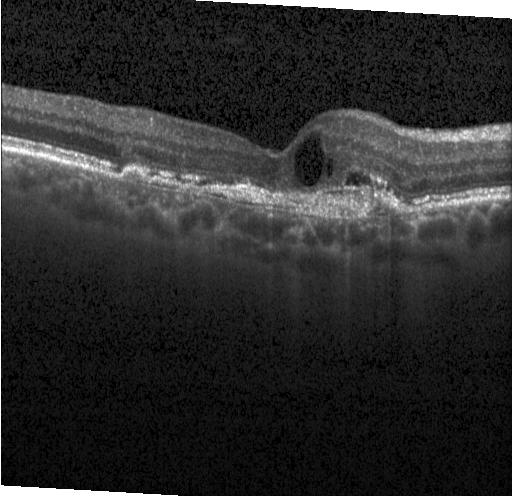 Retinal OCT cross-section. A choroidal neovascular membrane.